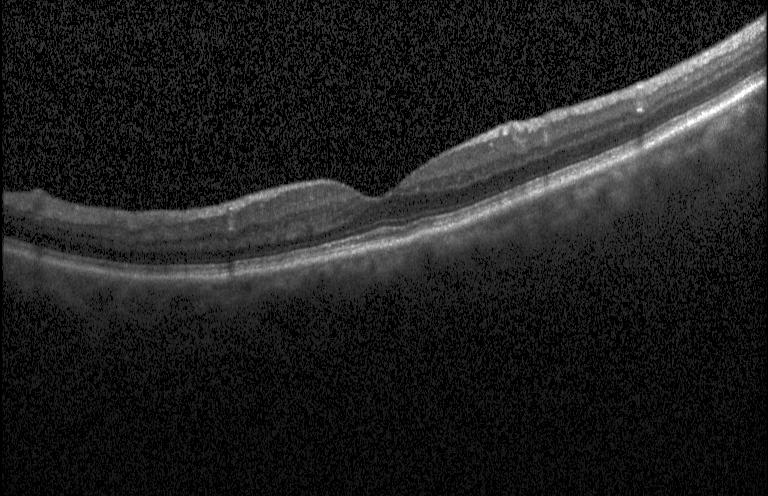
Retinal OCT cross-section showing no evidence of choroidal neovascularization, diabetic macular edema, or drusen.